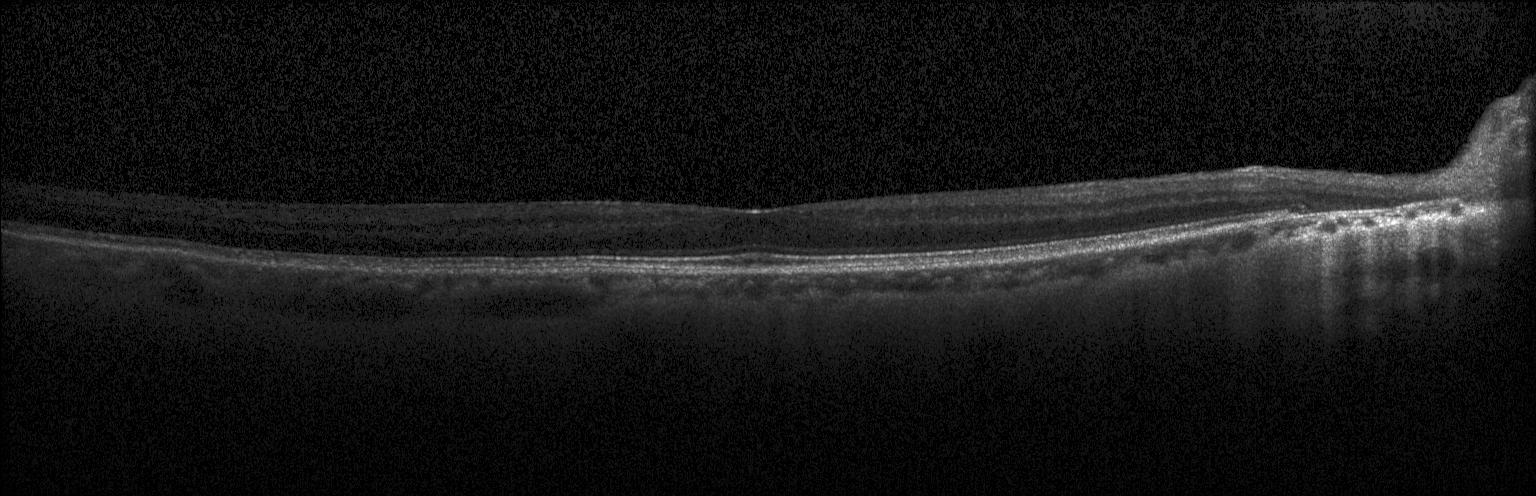

Finding: neither choroidal neovascularization, diabetic macular edema, nor drusen.